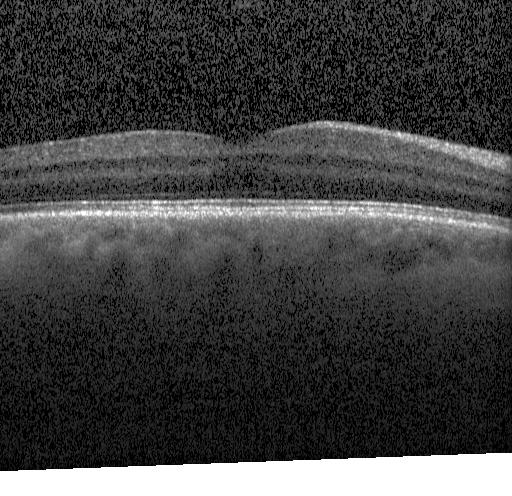

Heidelberg Spectralis. Through the macula. Optical coherence tomography scan. Spectral-domain optical coherence tomography — Diagnosis: neither CNV, DME, nor drusen.